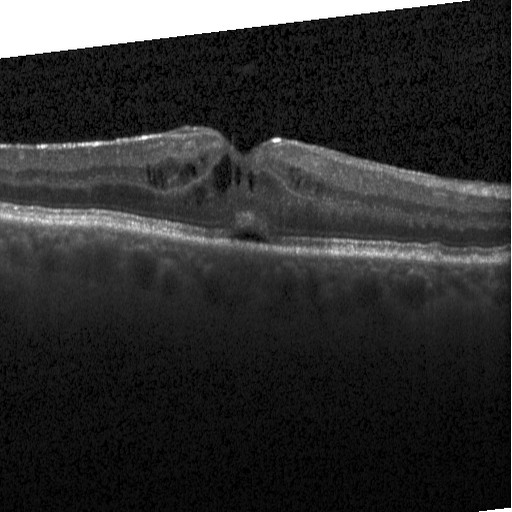 Macular scan. Retinal OCT cross-section. Acquired on a Heidelberg Spectralis. Impression: diabetic macular edema.